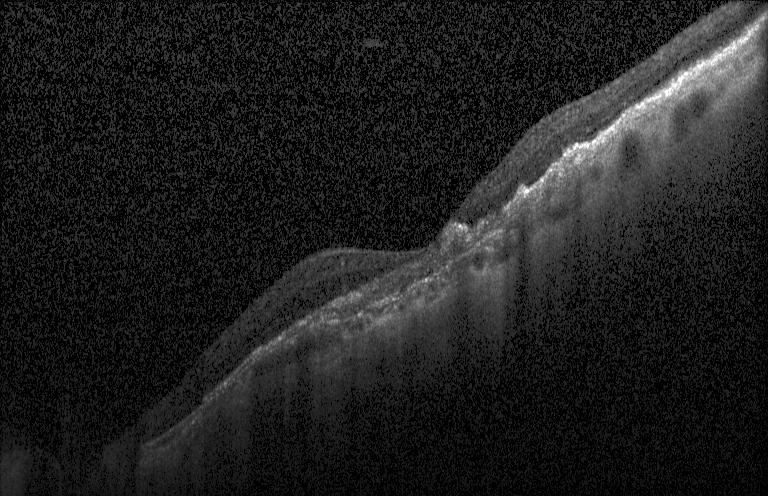 OCT B-scan
A choroidal neovascular membrane.